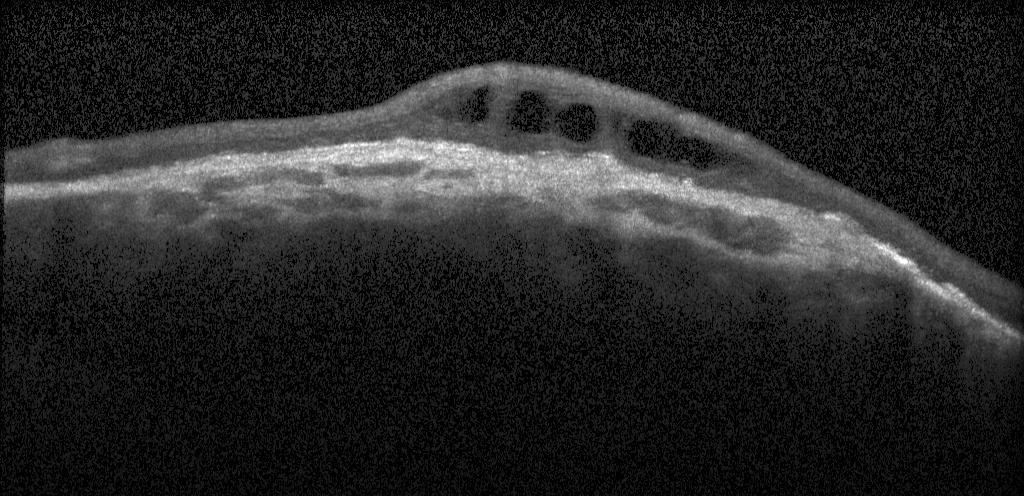

Fovea-centered. Optical coherence tomography B-scan. The scan shows a choroidal neovascular membrane.